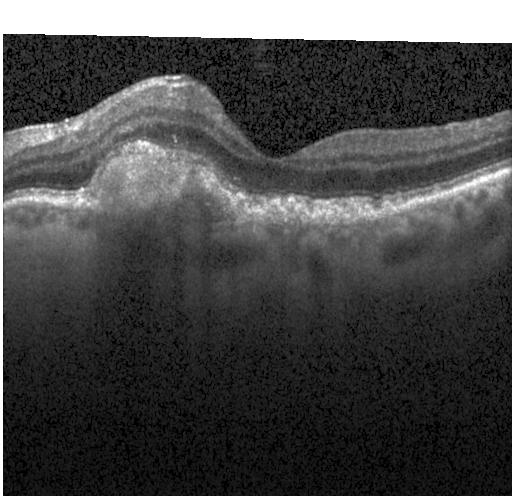 Diagnosis: a choroidal neovascular membrane.